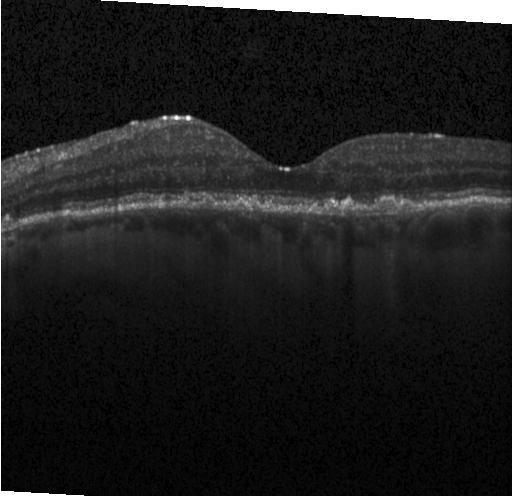
OCT line scan. Spectral-domain OCT. Horizontal scan through the fovea. This B-scan demonstrates multiple drusen.